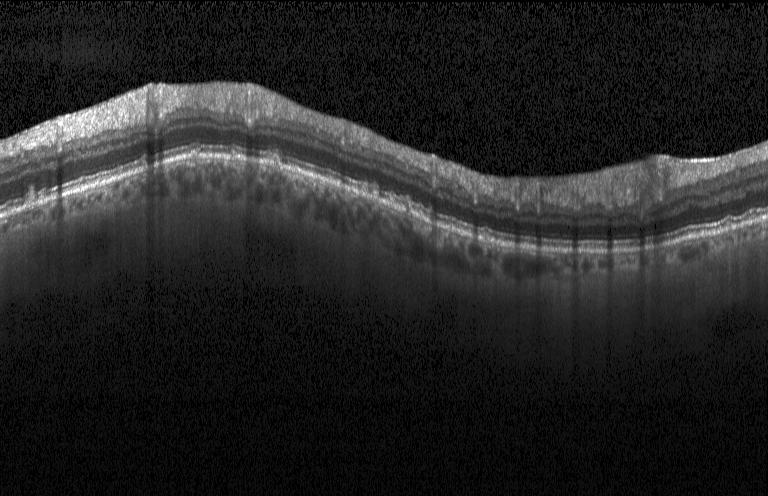

Sub-RPE drusenoid deposits.